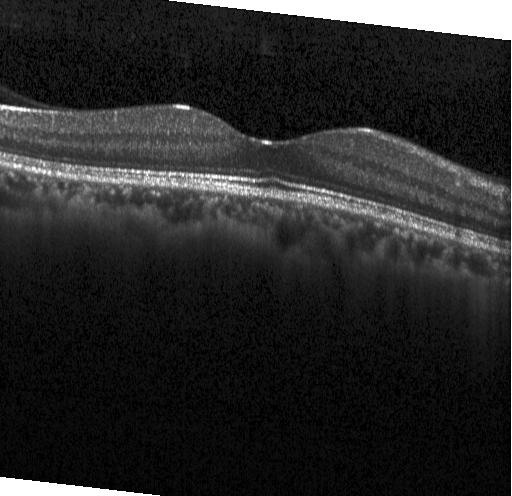
Instrument: Heidelberg Spectralis. Optical coherence tomography scan.
Diagnosis: neither choroidal neovascularization, diabetic macular edema, nor drusen.